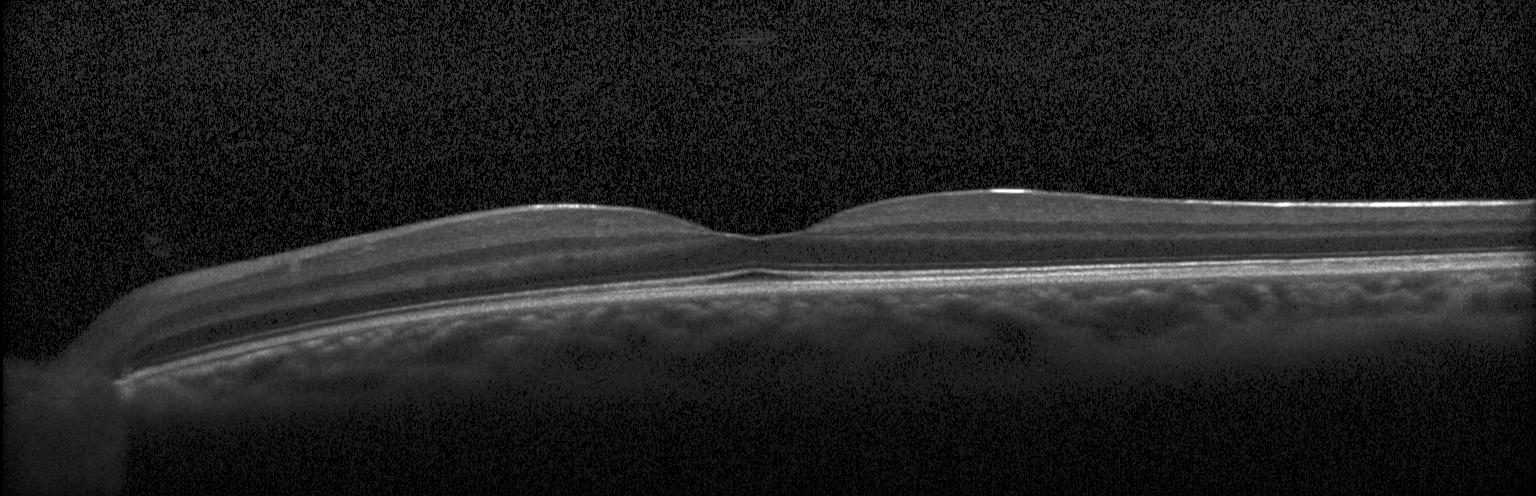

OCT finding: neither choroidal neovascularization, diabetic macular edema, nor drusen.